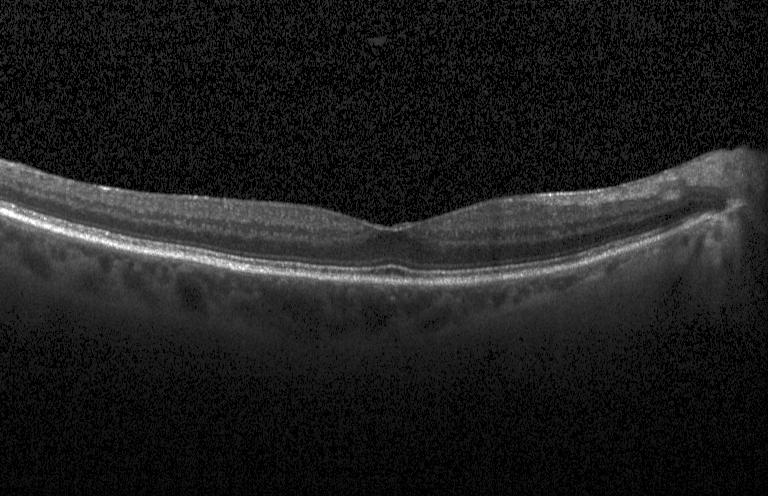

Heidelberg Spectralis OCT system · retinal OCT cross-section · through the macula.
Impression: no choroidal neovascularization, diabetic macular edema, or drusen.